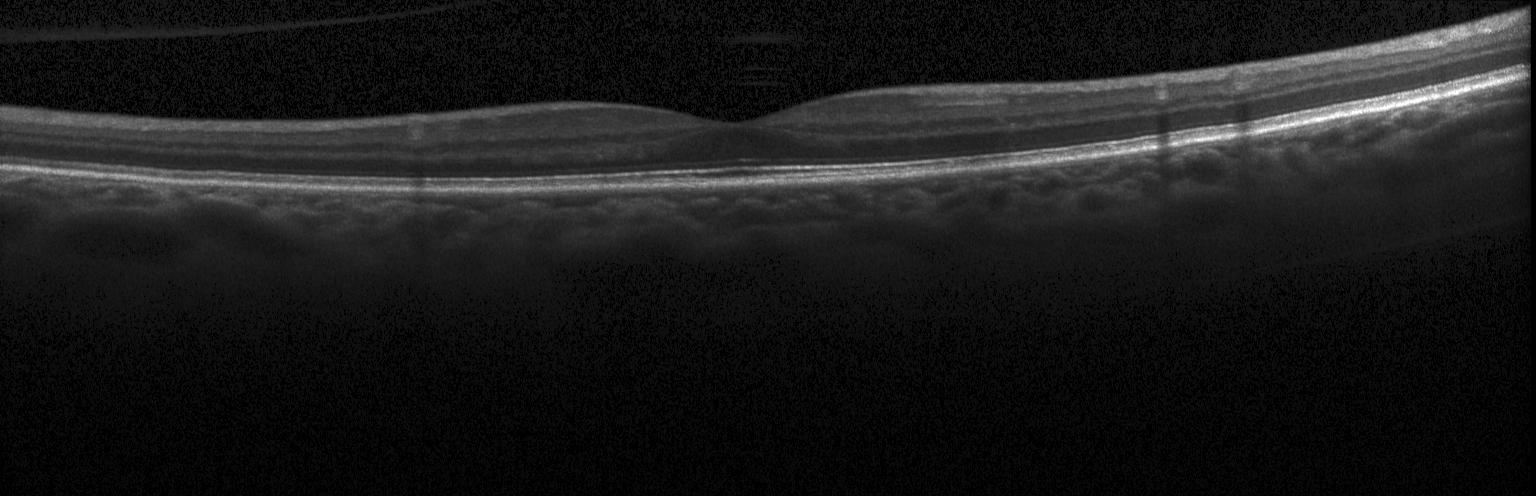 OCT line scan; centered on the fovea; Heidelberg Spectralis; SD-OCT
OCT finding: no evidence of choroidal neovascularization, diabetic macular edema, or drusen.